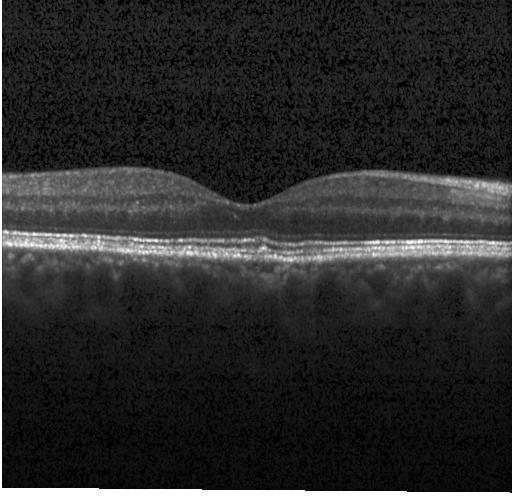 Retinal OCT B-scan. Spectral-domain OCT.
Impression: drusen.